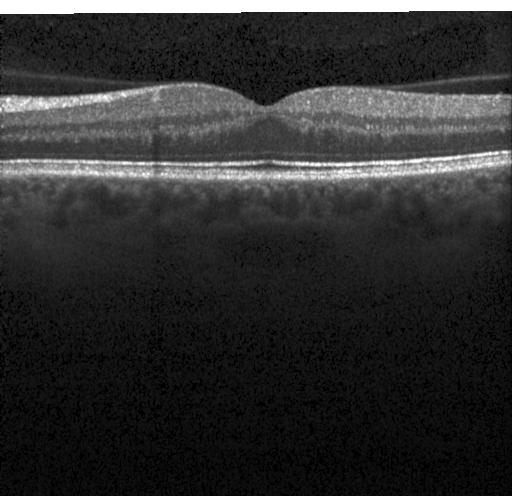 Retinal OCT cross-section showing no CNV, DME, or drusen.